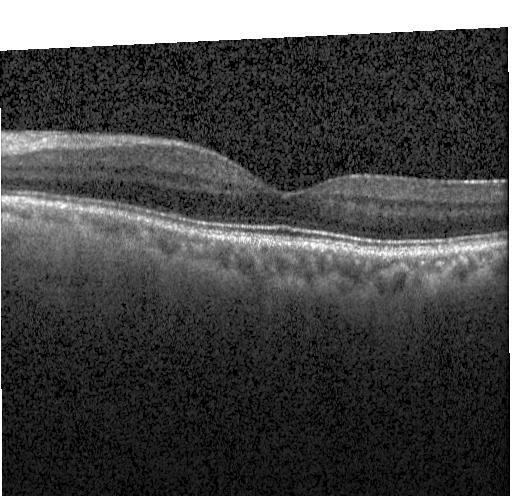
Spectral-domain OCT; retinal OCT cross-section; Heidelberg Spectralis — Finding: no choroidal neovascularization, no diabetic macular edema, and no drusen.